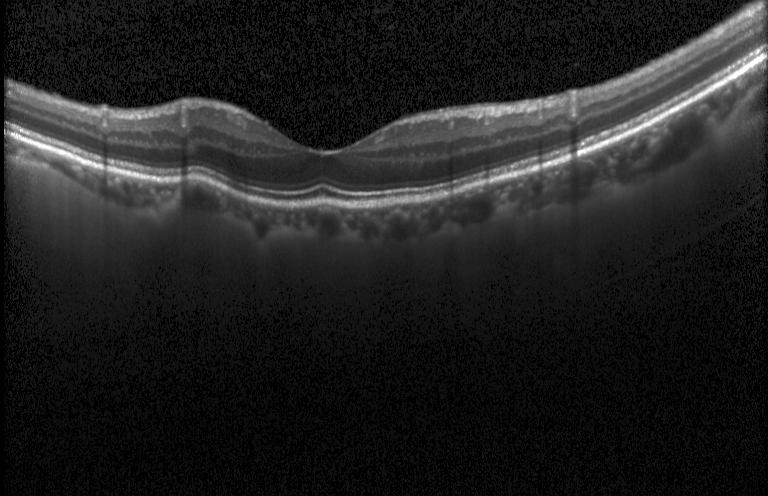
Assessment: no evidence of CNV, DME, or drusen.